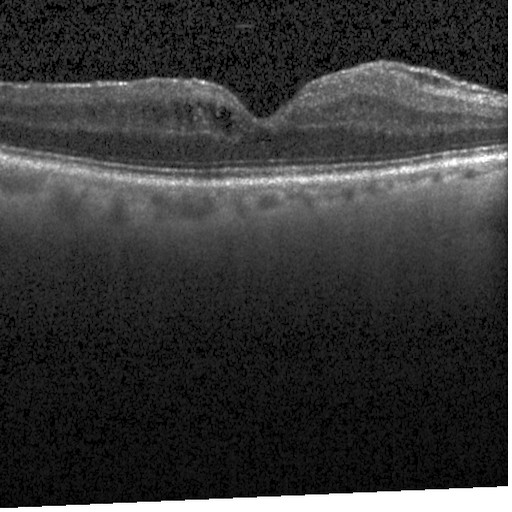
Retinal OCT B-scan. Impression: diabetic macular edema.